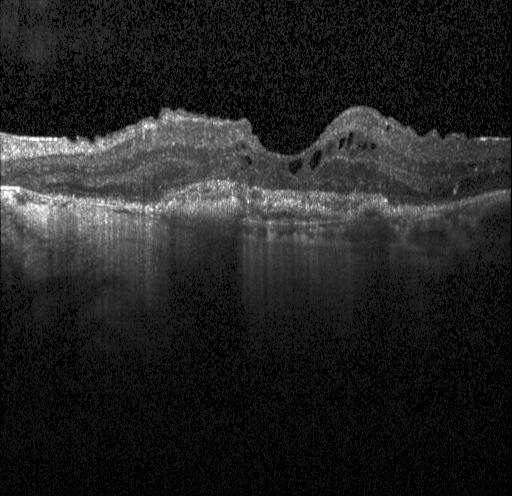
Spectral-domain optical coherence tomography, optical coherence tomography B-scan
Dx: choroidal neovascularization (CNV).